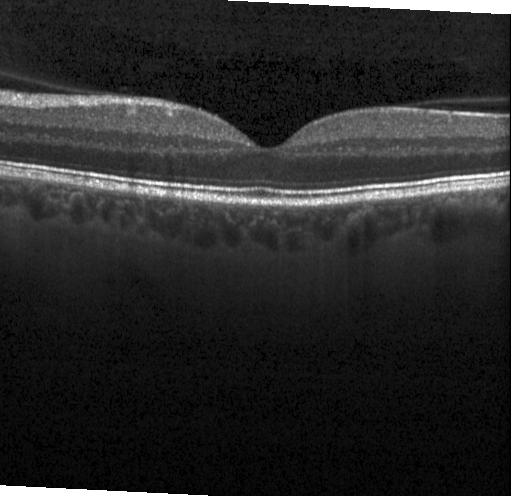
Retinal OCT B-scan. No evidence of CNV, DME, or drusen.